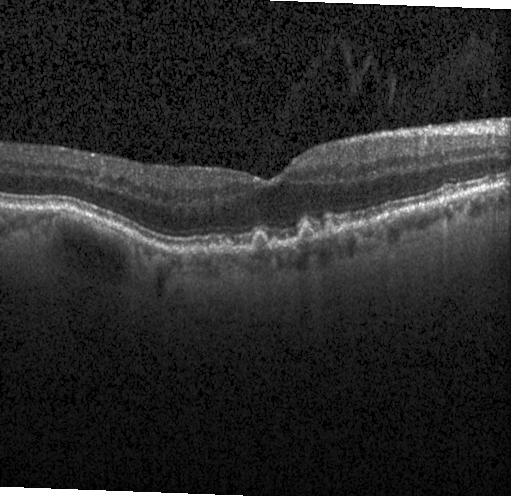
Drusen.